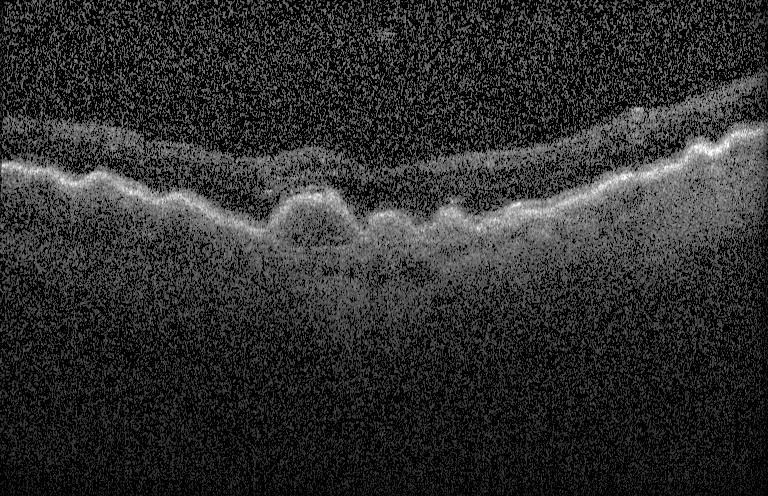 Retinal OCT B-scan, spectral-domain optical coherence tomography
Impression: a choroidal neovascular membrane.